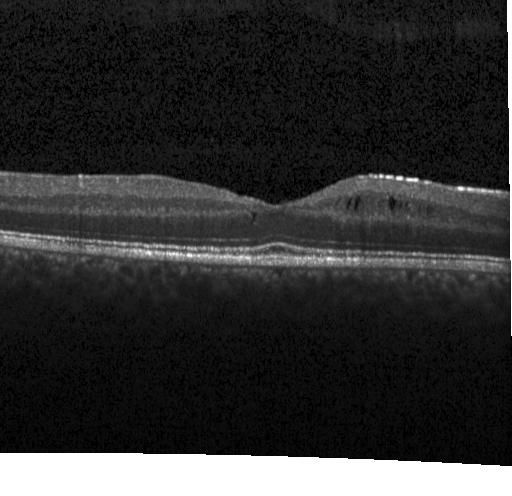 Spectral-domain OCT; instrument: Heidelberg Spectralis; retinal OCT cross-section; centered on the fovea — This B-scan demonstrates diabetic macular edema (DME).